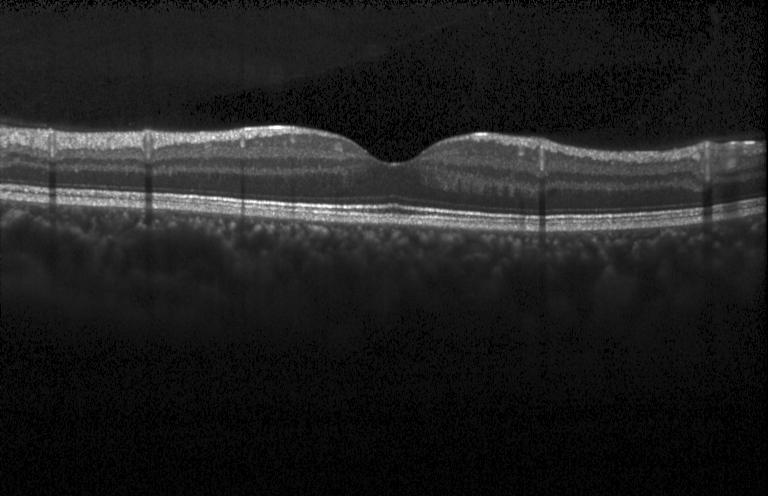
Retinal OCT B-scan; macular scan.
Impression: no choroidal neovascularization, diabetic macular edema, or drusen.